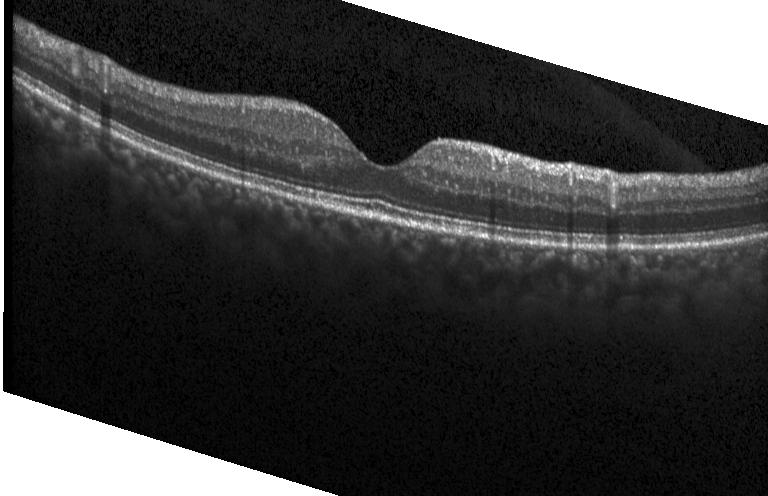
OCT line scan
Finding: no CNV, no DME, and no drusen.